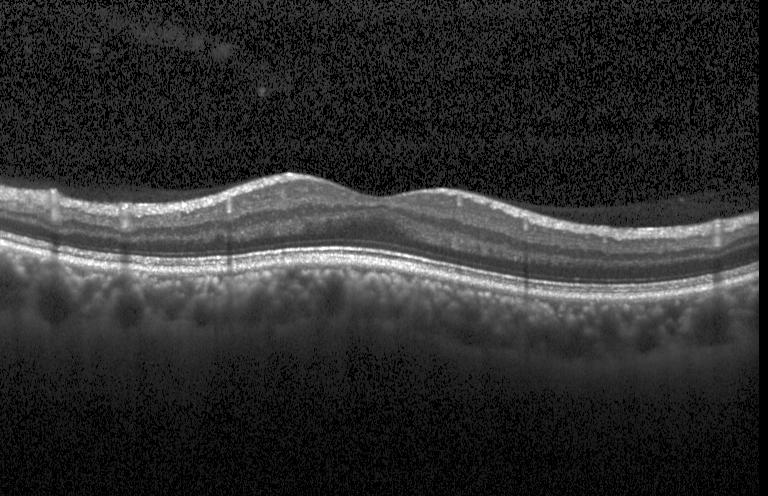
Acquired on a Heidelberg Spectralis · retinal OCT cross-section
Assessment: no evidence of choroidal neovascularization, diabetic macular edema, or drusen.